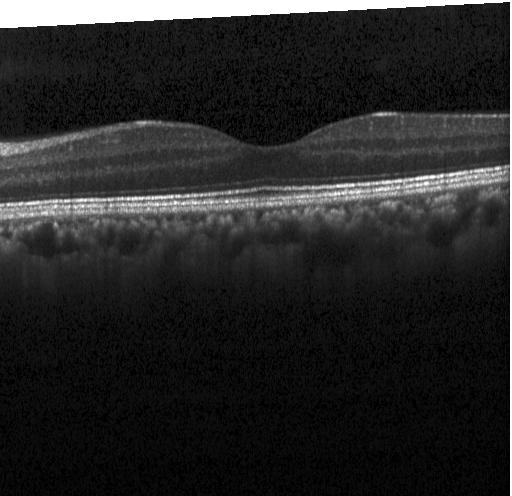
Macular scan · SD-OCT · optical coherence tomography B-scan — Dx: no choroidal neovascularization, diabetic macular edema, or drusen.